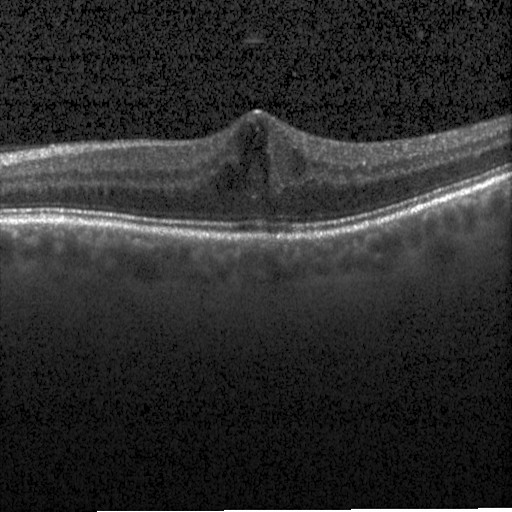
Optical coherence tomography B-scan · Heidelberg Spectralis · centered on the fovea · spectral-domain optical coherence tomography
Impression: DME.